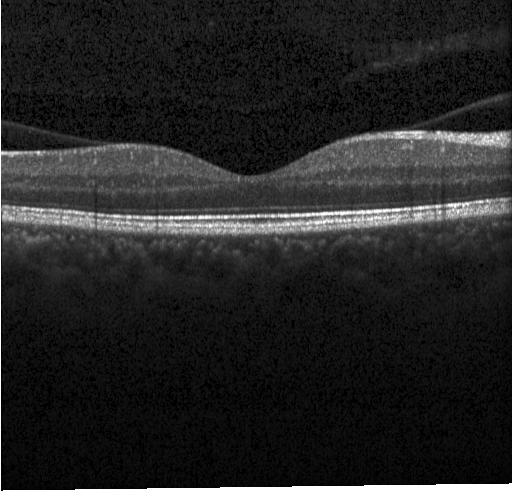 Centered on the fovea · optical coherence tomography B-scan · Heidelberg Spectralis · SD-OCT.
Impression: neither choroidal neovascularization, diabetic macular edema, nor drusen.